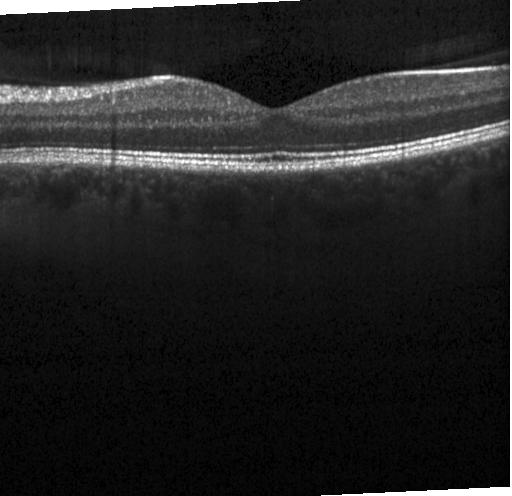

Retinal OCT B-scan. Horizontal scan through the fovea. Acquired on a Heidelberg Spectralis — No choroidal neovascularization, no diabetic macular edema, and no drusen.